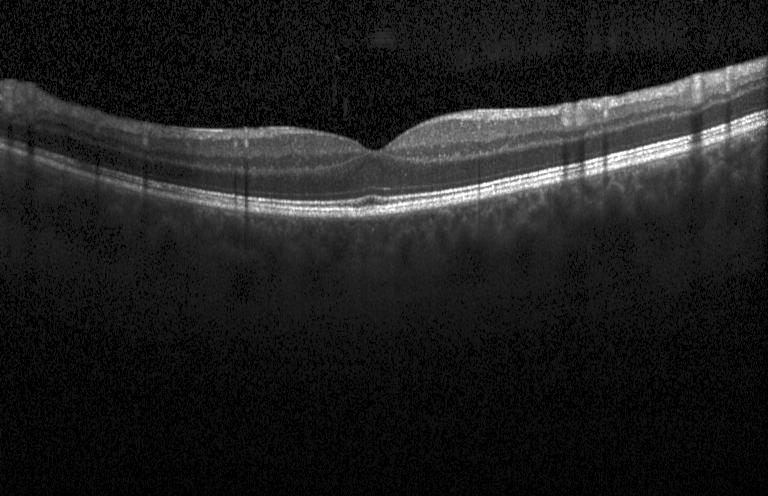

OCT scan showing neither choroidal neovascularization, diabetic macular edema, nor drusen.